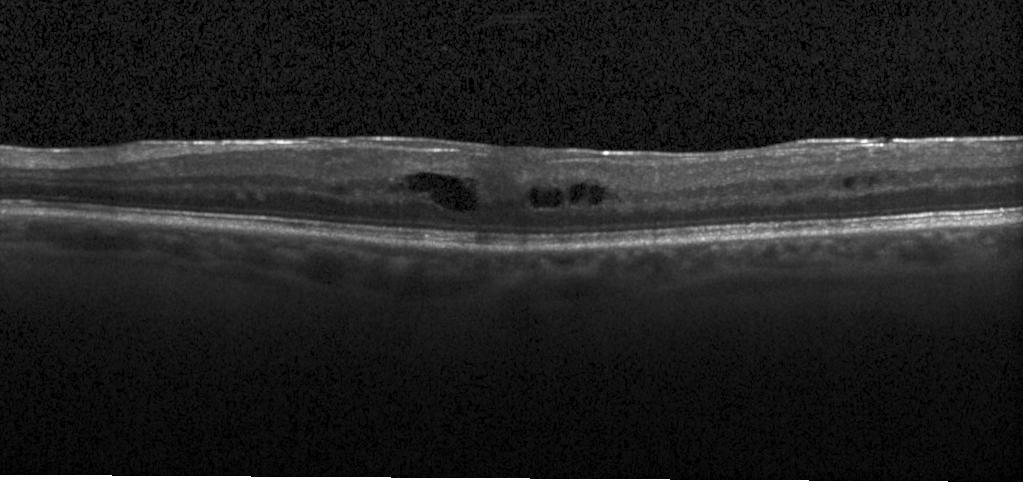 Optical coherence tomography scan — This B-scan demonstrates DME.